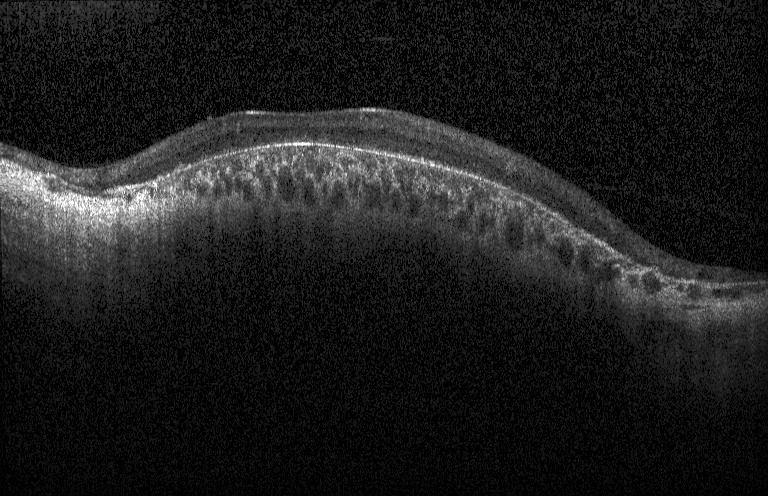
Optical coherence tomography scan. SD-OCT
Finding: neither CNV, DME, nor drusen.